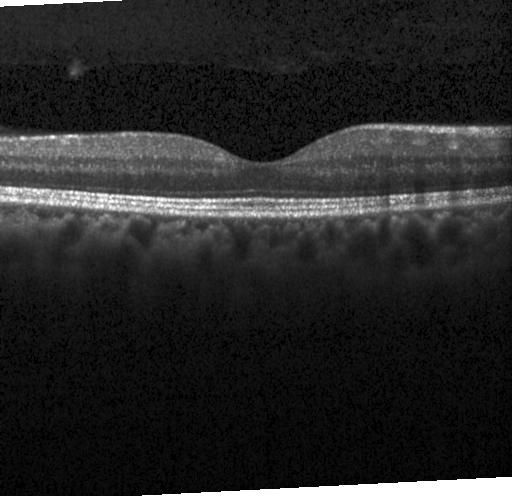
Fovea-centered; optical coherence tomography B-scan; Heidelberg Spectralis OCT system.
Macular OCT: no evidence of CNV, DME, or drusen.